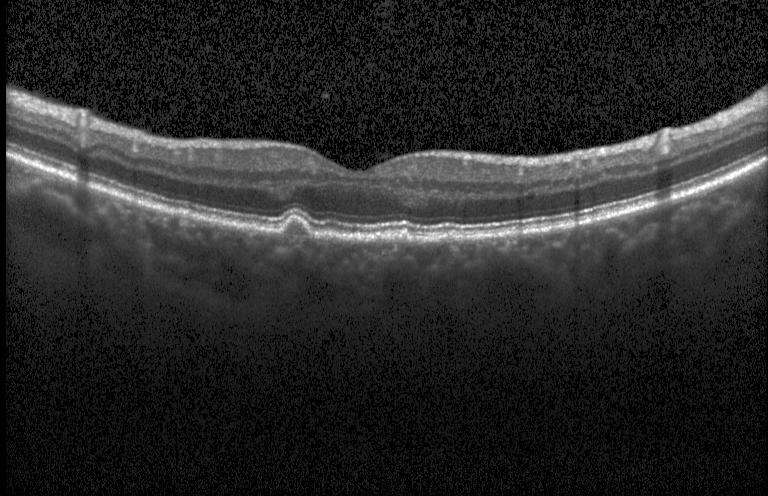
Diagnosis: sub-RPE drusenoid deposits.